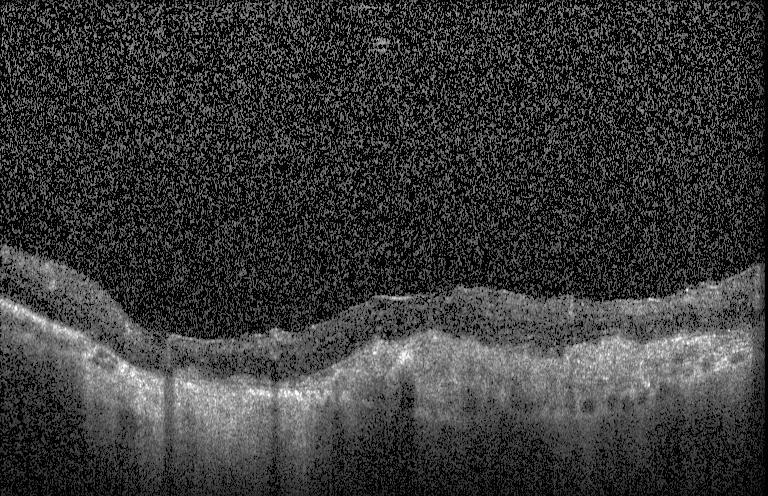 Optical coherence tomography scan — Diagnosis: CNV.